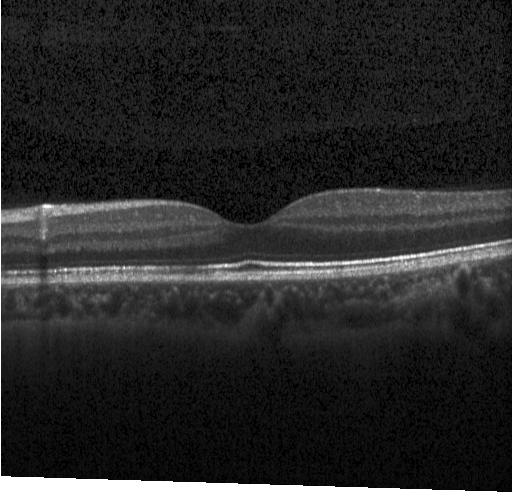

Diagnosis: no choroidal neovascularization, diabetic macular edema, or drusen.